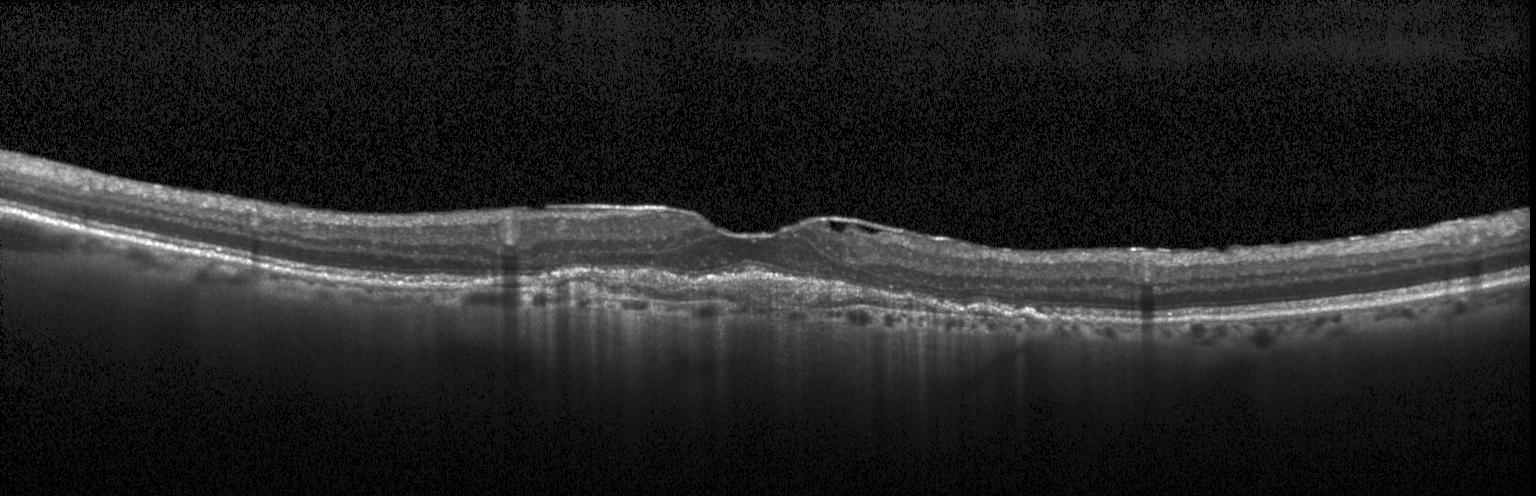
Through the macula · retinal OCT B-scan.
Diagnosis: CNV.